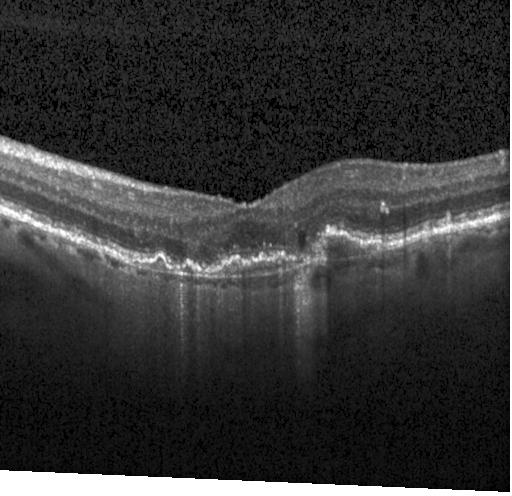
Spectral-domain optical coherence tomography; OCT B-scan; macular scan; Heidelberg Spectralis.
Impression: choroidal neovascularization (CNV).